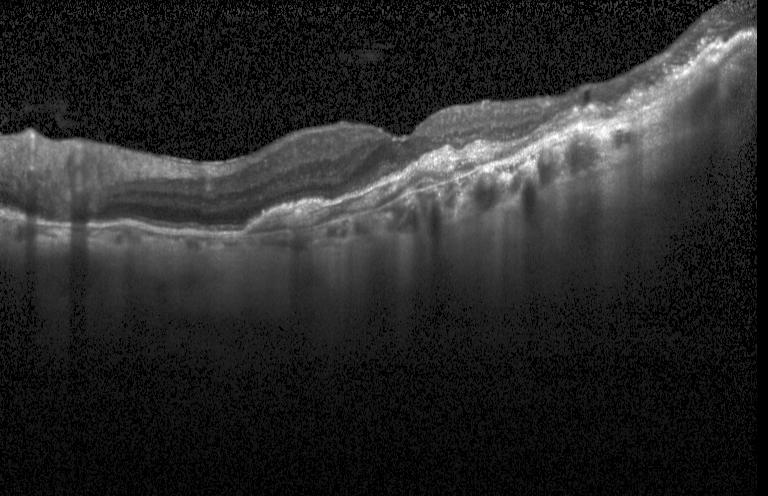
Heidelberg Spectralis OCT system, fovea-centered, retinal OCT cross-section.
Impression: a choroidal neovascular membrane.